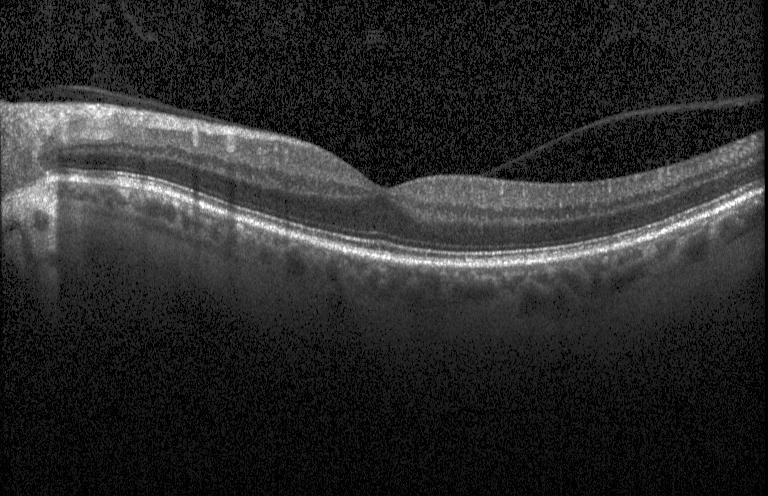
OCT line scan · Heidelberg Spectralis. Assessment: neither choroidal neovascularization, diabetic macular edema, nor drusen.